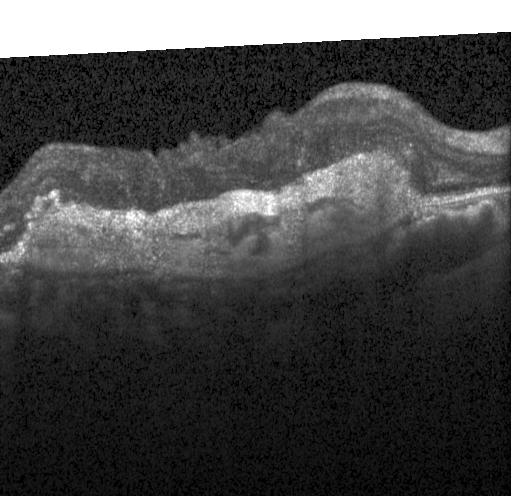

Optical coherence tomography B-scan — Diagnosis: CNV.